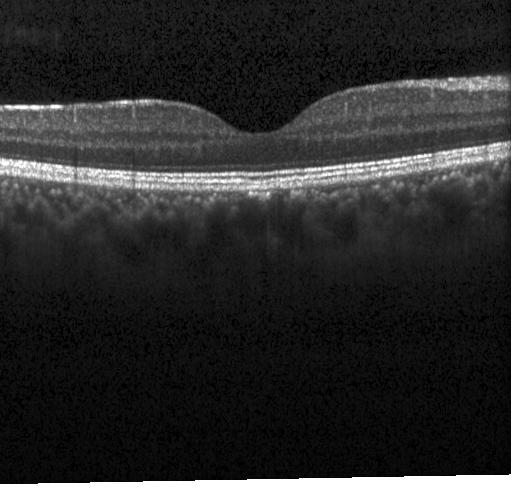
Finding: neither choroidal neovascularization, diabetic macular edema, nor drusen.